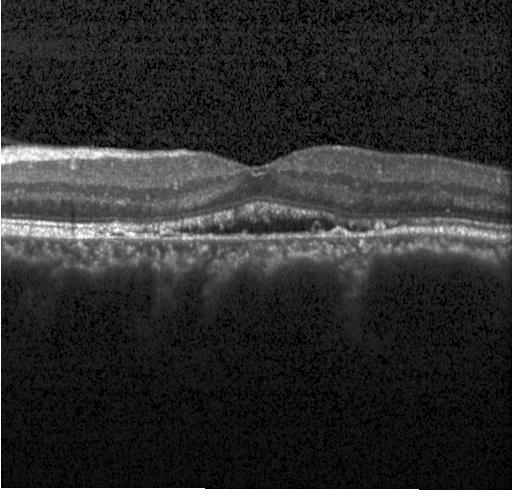 Through the macula. Acquired on a Heidelberg Spectralis. SD-OCT. Optical coherence tomography B-scan
Dx: CNV.